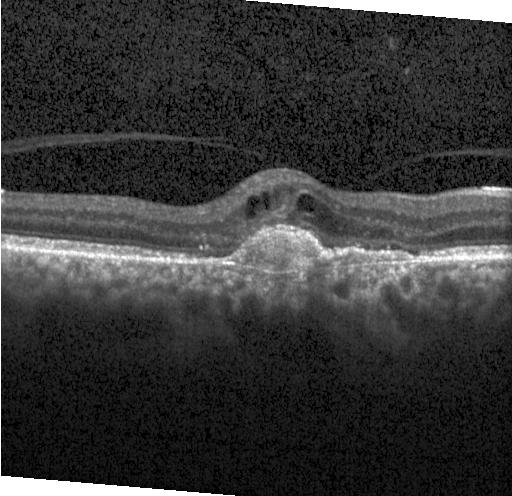
Retinal OCT cross-section showing a choroidal neovascular membrane.